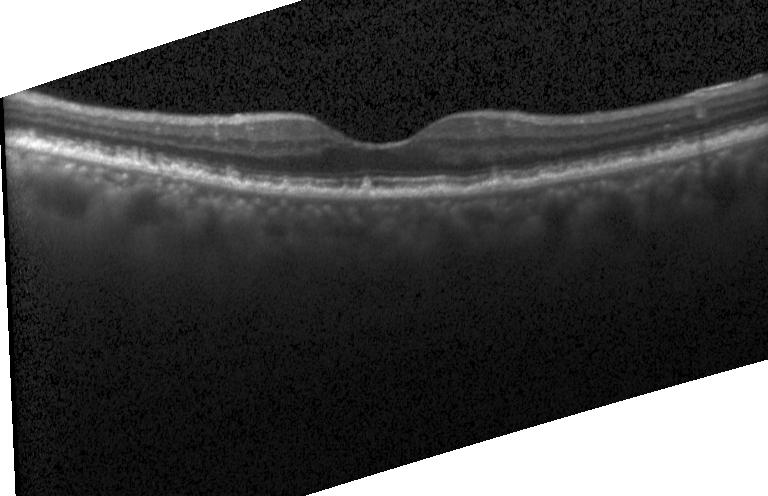

This B-scan demonstrates multiple drusen.